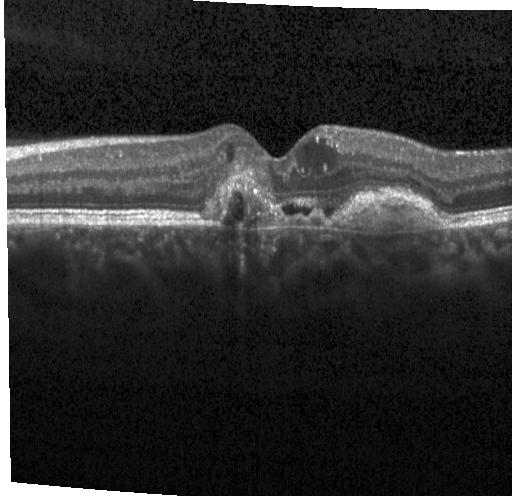

The scan shows CNV.